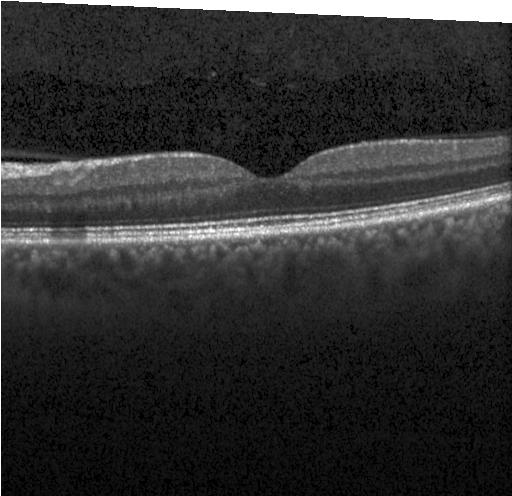

Macular scan, Heidelberg Spectralis, OCT B-scan
This B-scan demonstrates no choroidal neovascularization, diabetic macular edema, or drusen.